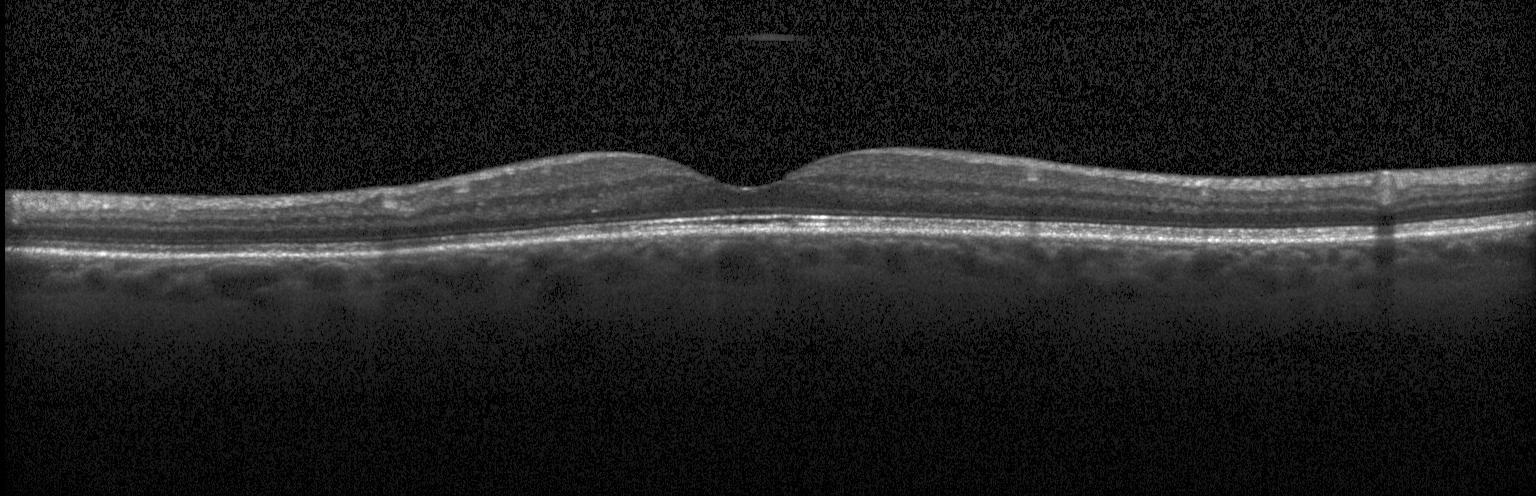

Dx: no choroidal neovascularization, diabetic macular edema, or drusen.